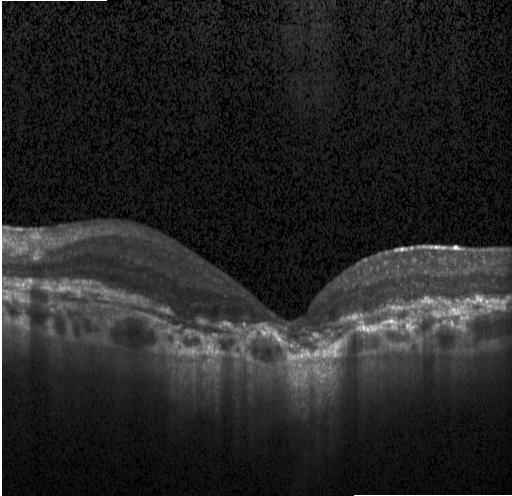

OCT B-scan showing choroidal neovascularization (CNV).